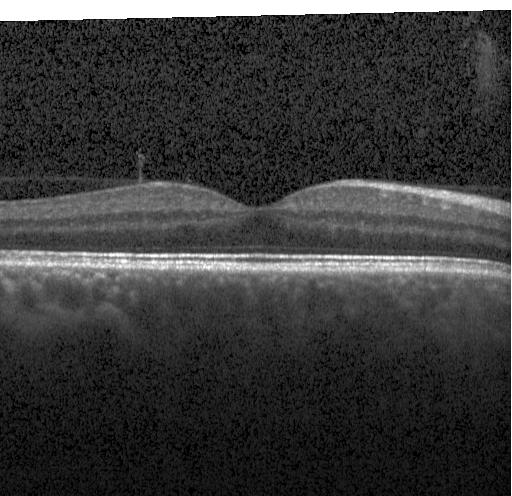 Optical coherence tomography scan — OCT finding: no evidence of CNV, DME, or drusen.